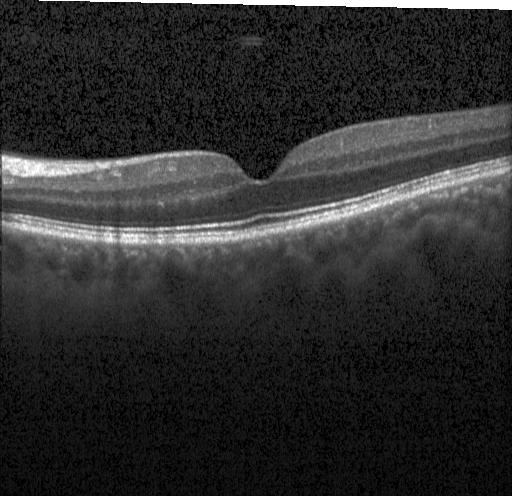 Spectral-domain optical coherence tomography · optical coherence tomography B-scan · centered on the fovea · Heidelberg Spectralis
Impression: no choroidal neovascularization, no diabetic macular edema, and no drusen.